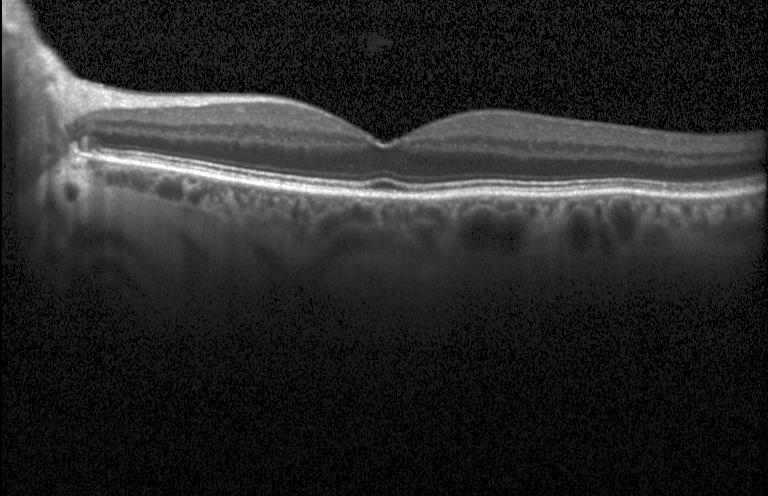

Impression: neither choroidal neovascularization, diabetic macular edema, nor drusen.